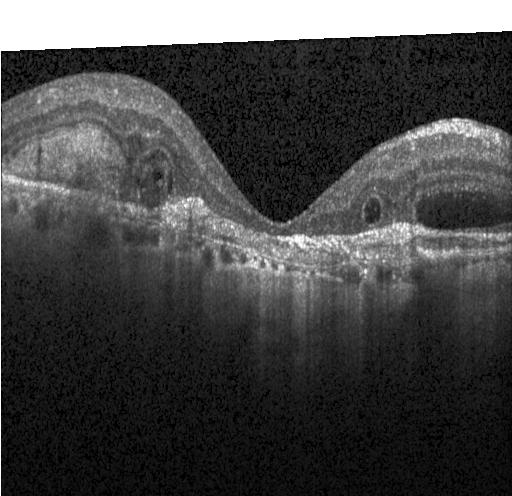

OCT B-scan, through the macula. The scan shows a choroidal neovascular membrane.